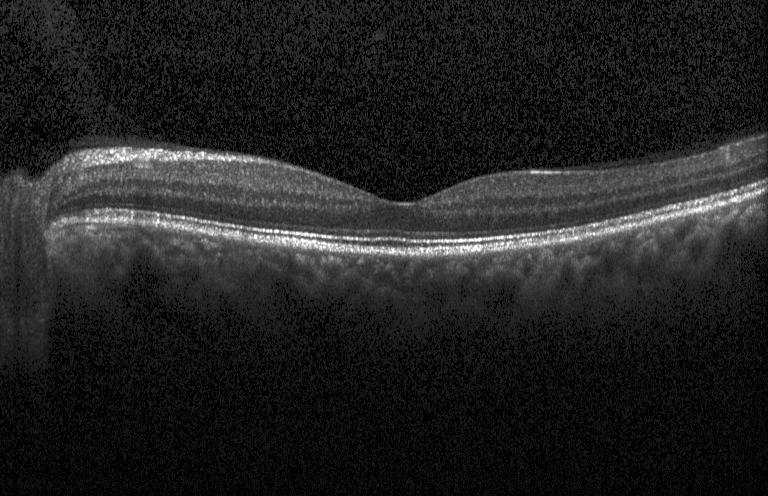

Impression: neither choroidal neovascularization, diabetic macular edema, nor drusen.